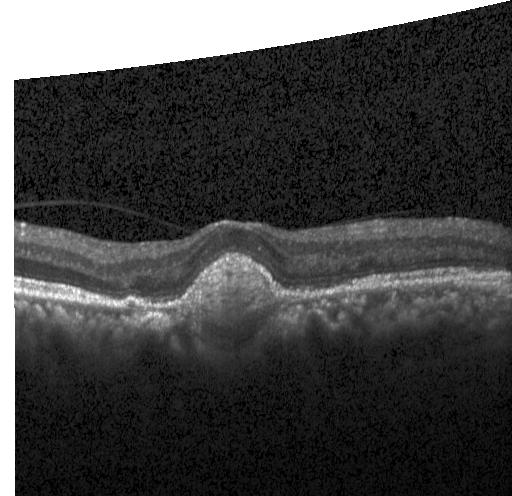
OCT line scan; horizontal scan through the fovea; SD-OCT; acquired on a Heidelberg Spectralis
Dx: CNV.